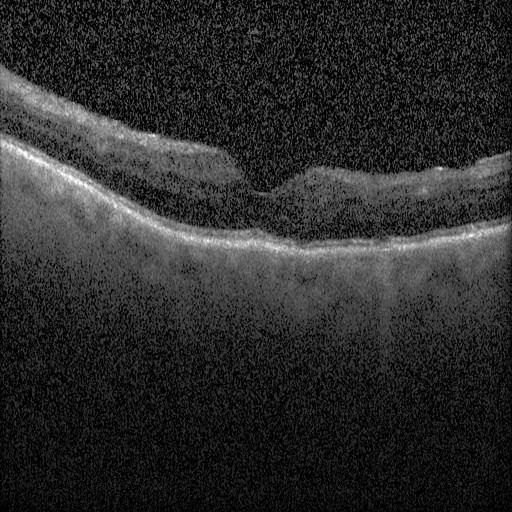

OCT scan showing diabetic macular edema (DME).